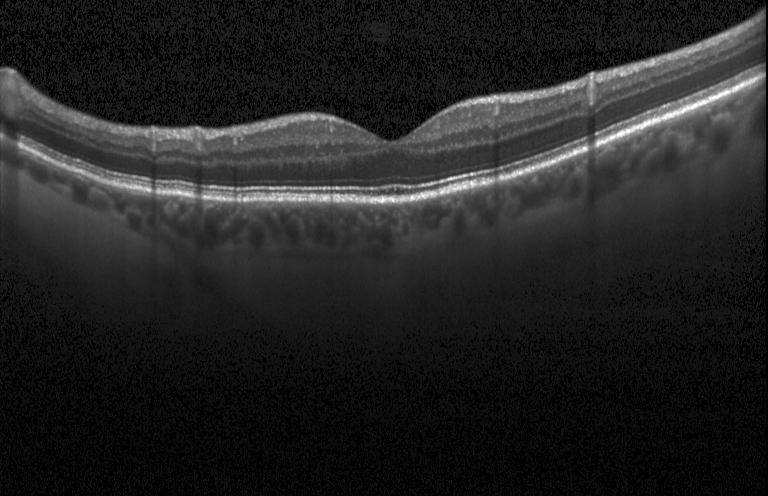

OCT B-scan showing no choroidal neovascularization, no diabetic macular edema, and no drusen.